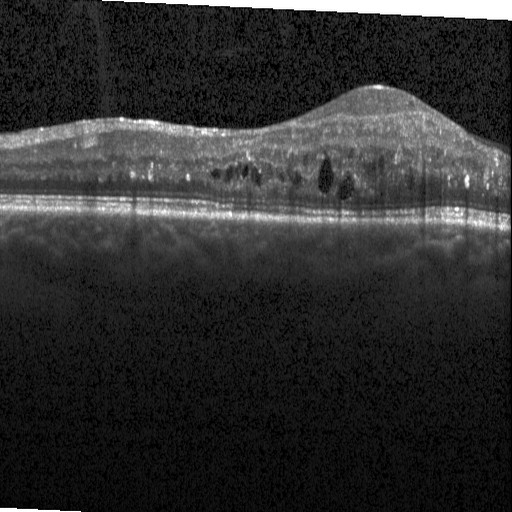 Retinal OCT B-scan, horizontal scan through the fovea. OCT finding: diabetic macular edema.